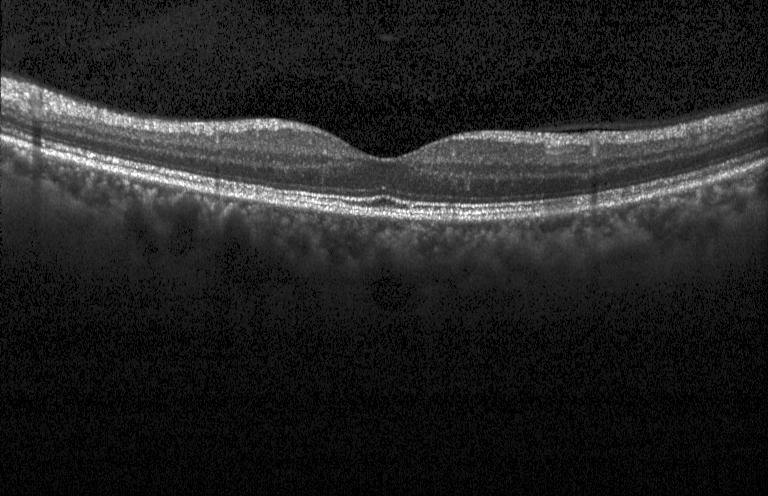 Instrument: Heidelberg Spectralis · OCT line scan — Diagnosis: no choroidal neovascularization, diabetic macular edema, or drusen.